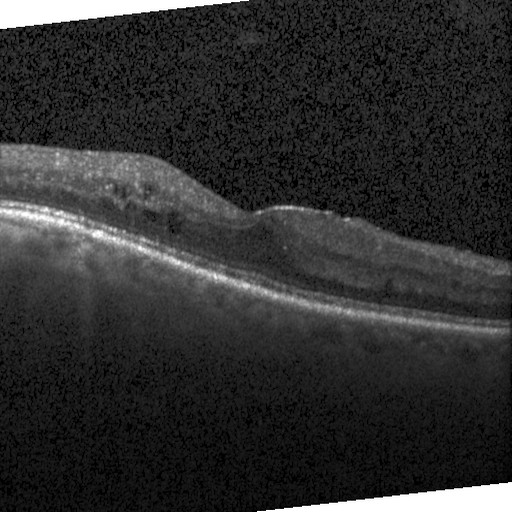
Retinal OCT B-scan.
Assessment: DME.